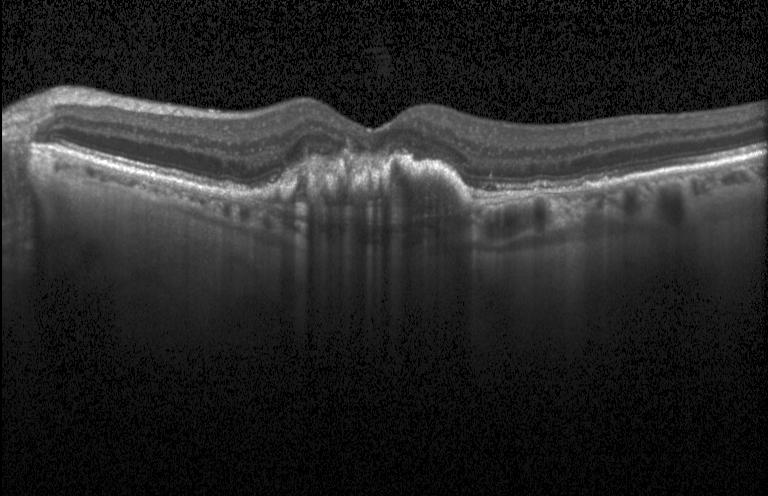
The scan shows a choroidal neovascular membrane.